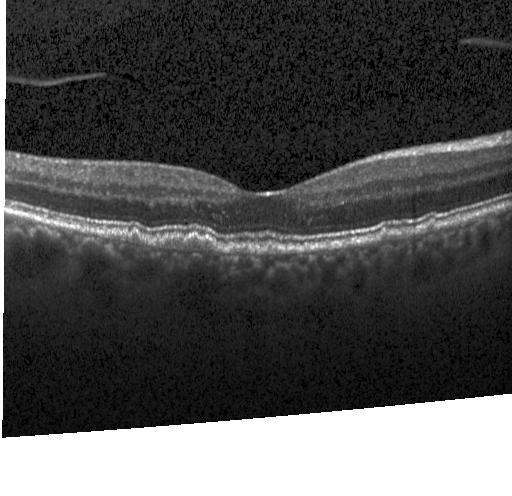 Retinal OCT B-scan; SD-OCT; Heidelberg Spectralis. Diagnosis: drusen.